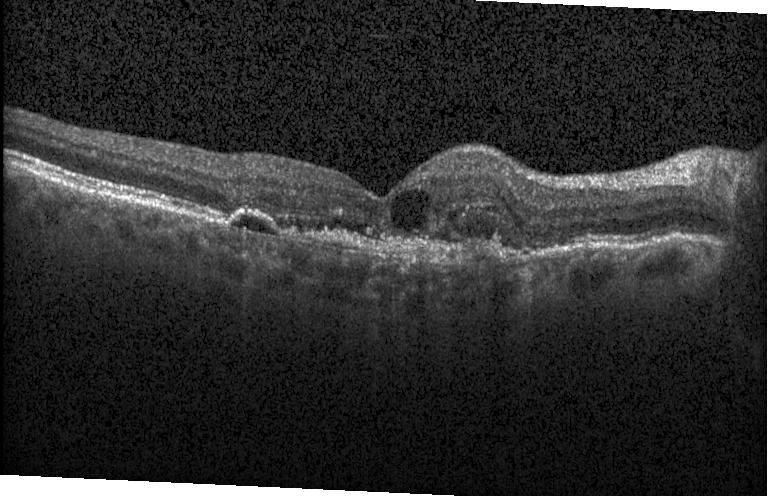
Retinal OCT cross-section showing a choroidal neovascular membrane.